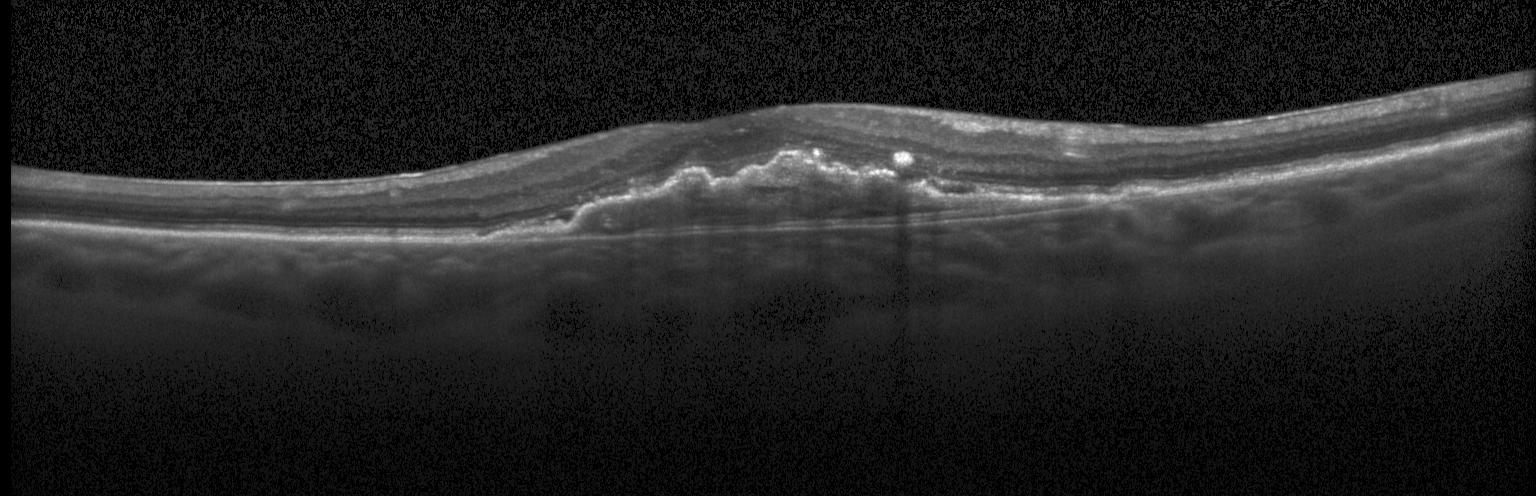
Fovea-centered · spectral-domain optical coherence tomography · OCT B-scan · instrument: Heidelberg Spectralis — Impression: choroidal neovascularization (CNV).